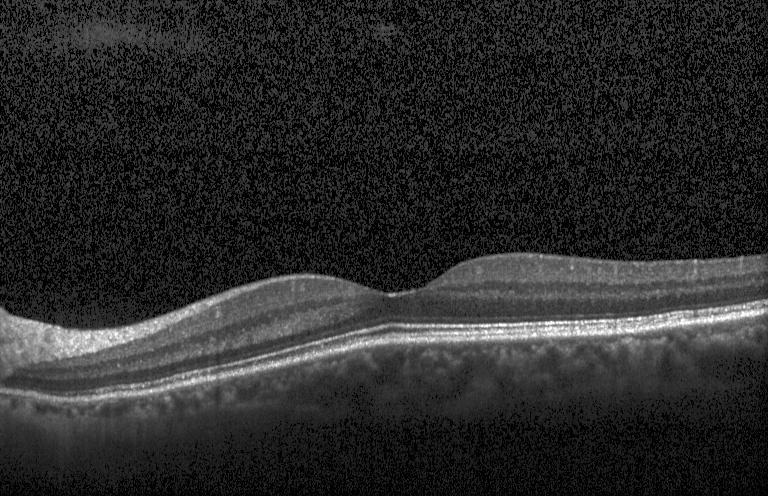 Finding: no evidence of CNV, DME, or drusen.